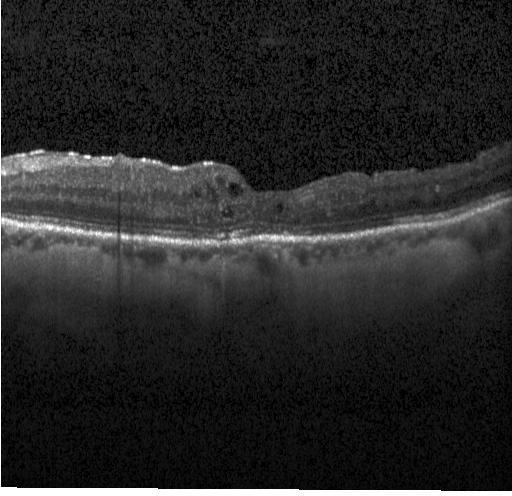

SD-OCT · acquired on a Heidelberg Spectralis · optical coherence tomography scan · fovea-centered.
Diagnosis: diabetic macular edema (DME).